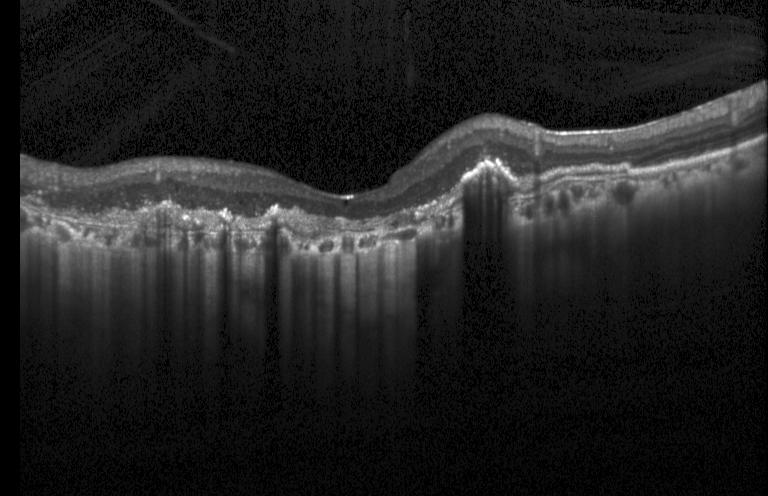
Optical coherence tomography scan. Spectral-domain OCT.
Finding: choroidal neovascularization (CNV).